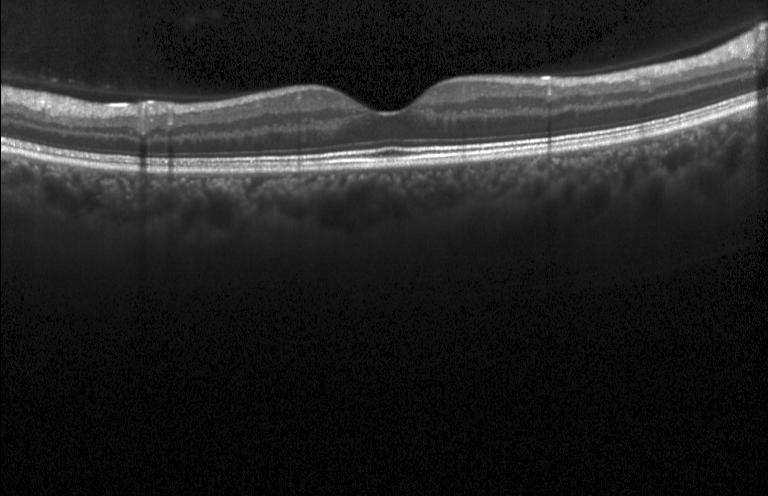 Neither choroidal neovascularization, diabetic macular edema, nor drusen.